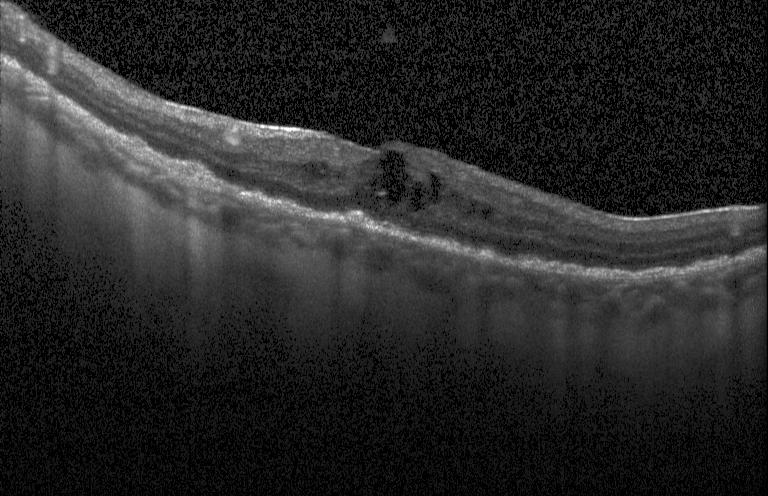
Optical coherence tomography scan — DME.